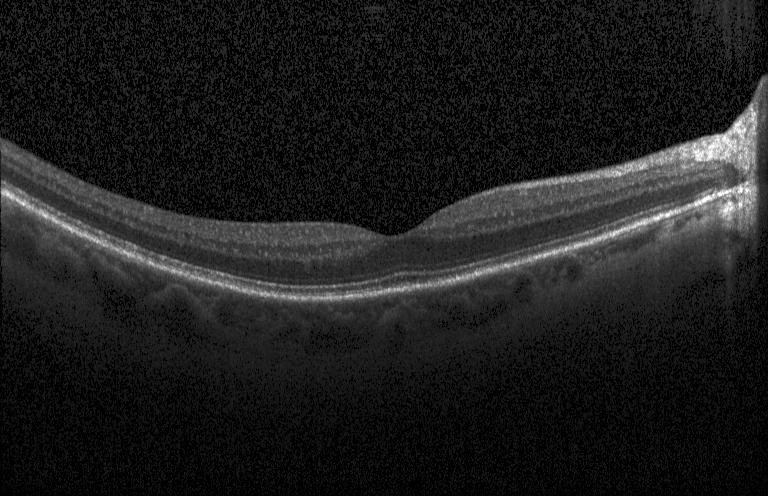
Diagnosis: neither CNV, DME, nor drusen.